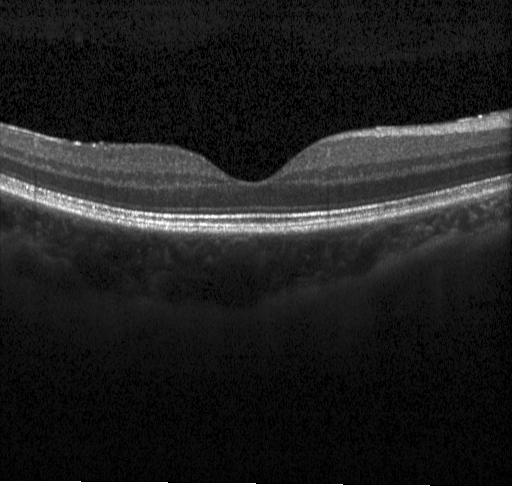 Optical coherence tomography B-scan — Impression: no choroidal neovascularization, no diabetic macular edema, and no drusen.